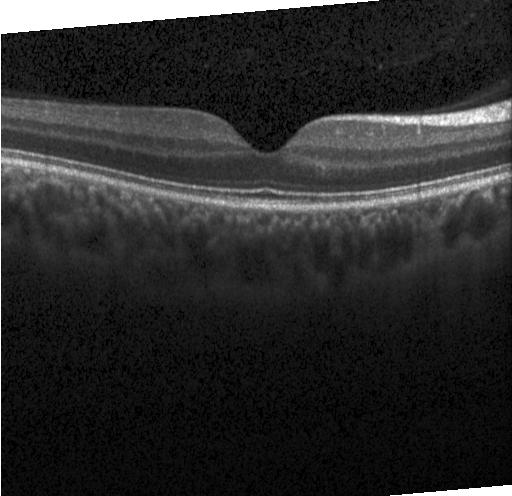
Optical coherence tomography scan — Assessment: no choroidal neovascularization, no diabetic macular edema, and no drusen.